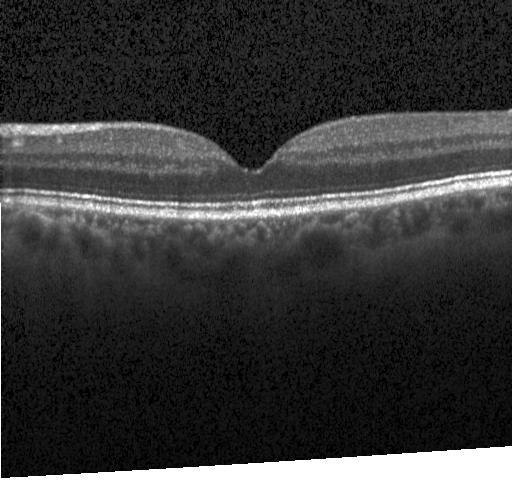
OCT scan showing neither choroidal neovascularization, diabetic macular edema, nor drusen.